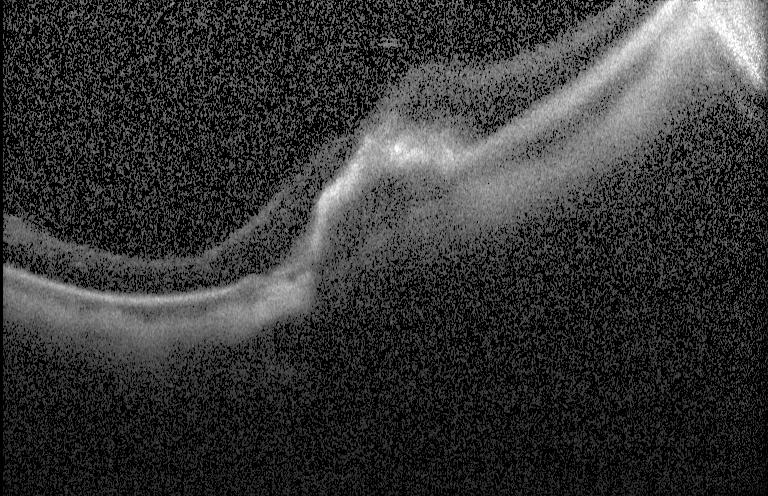
The scan shows a choroidal neovascular membrane.